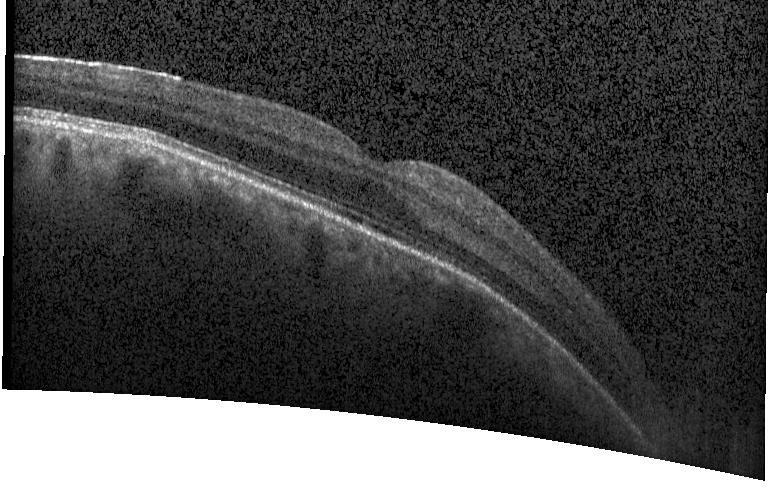 Horizontal scan through the fovea. Heidelberg Spectralis. SD-OCT. Optical coherence tomography B-scan — Impression: no evidence of choroidal neovascularization, diabetic macular edema, or drusen.